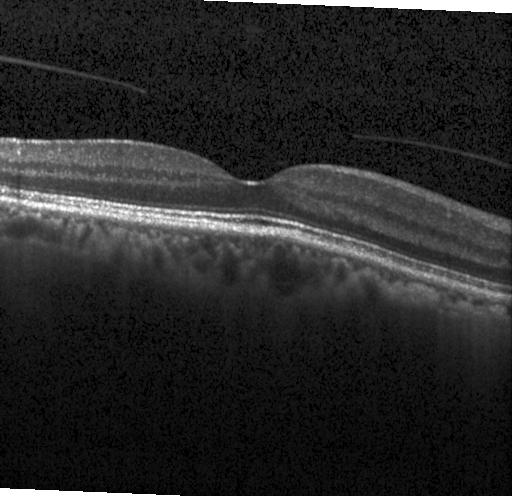
SD-OCT; retinal OCT B-scan.
No choroidal neovascularization, no diabetic macular edema, and no drusen.